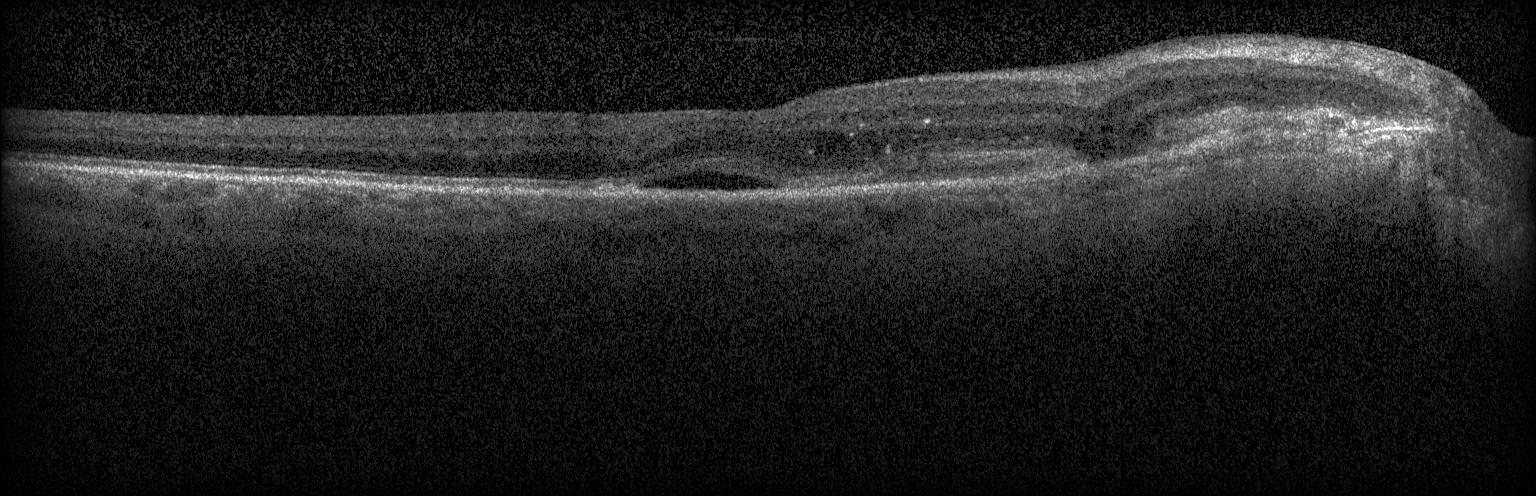 Optical coherence tomography B-scan.
A choroidal neovascular membrane.